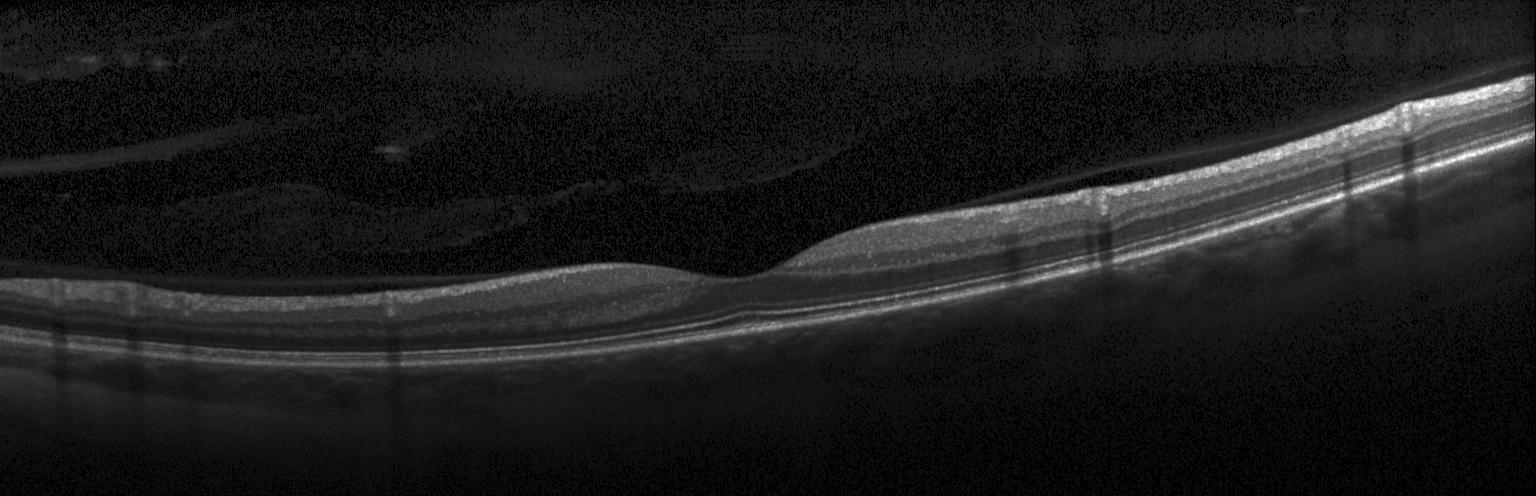
Horizontal scan through the fovea. Optical coherence tomography B-scan
OCT finding: no choroidal neovascularization, no diabetic macular edema, and no drusen.